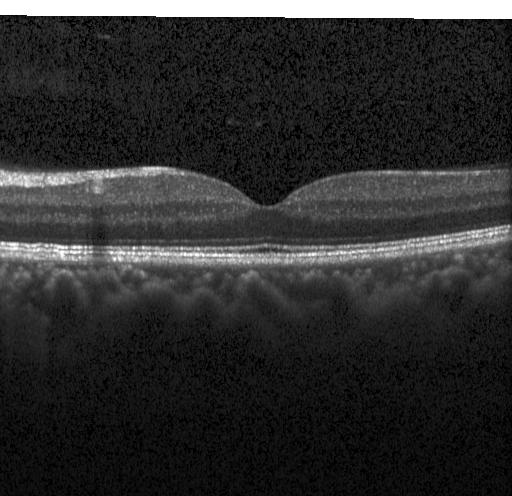
Through the macula. Spectral-domain OCT. Retinal OCT cross-section
Diagnosis: no evidence of choroidal neovascularization, diabetic macular edema, or drusen.